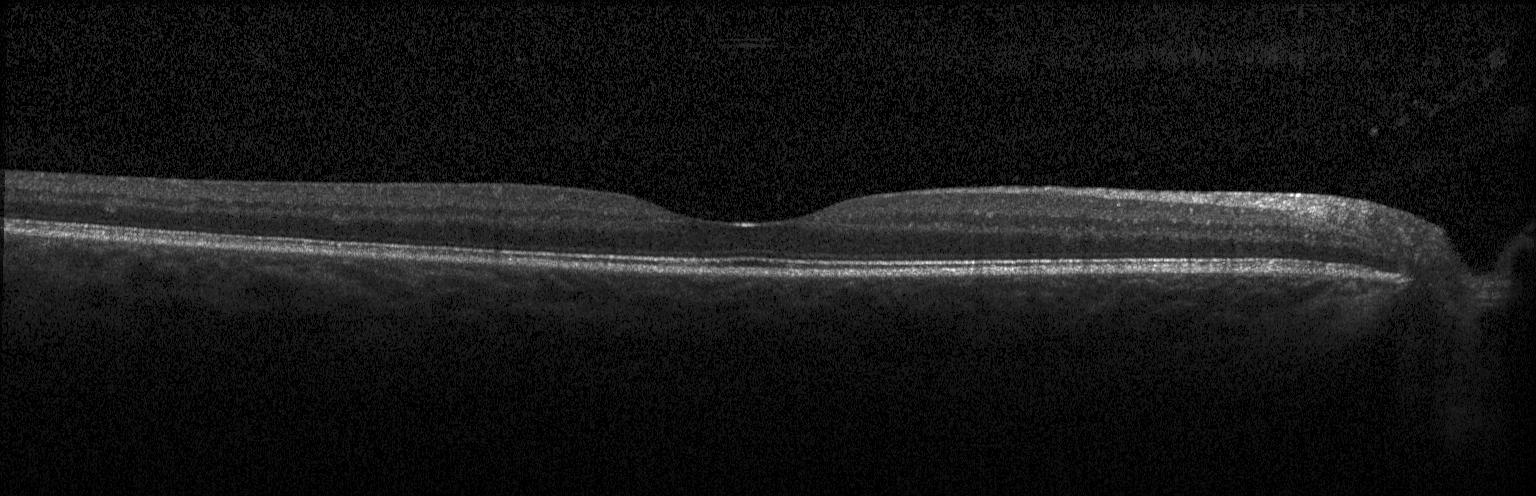

Heidelberg Spectralis OCT system, optical coherence tomography B-scan — Impression: no choroidal neovascularization, diabetic macular edema, or drusen.